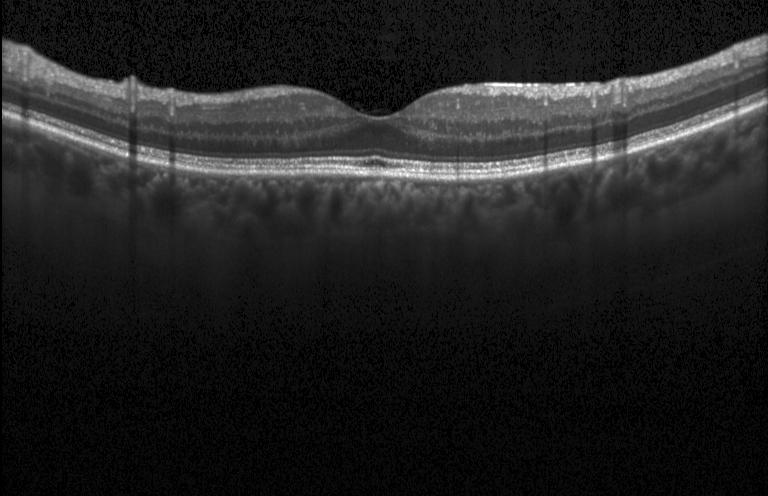

The scan shows no evidence of CNV, DME, or drusen.